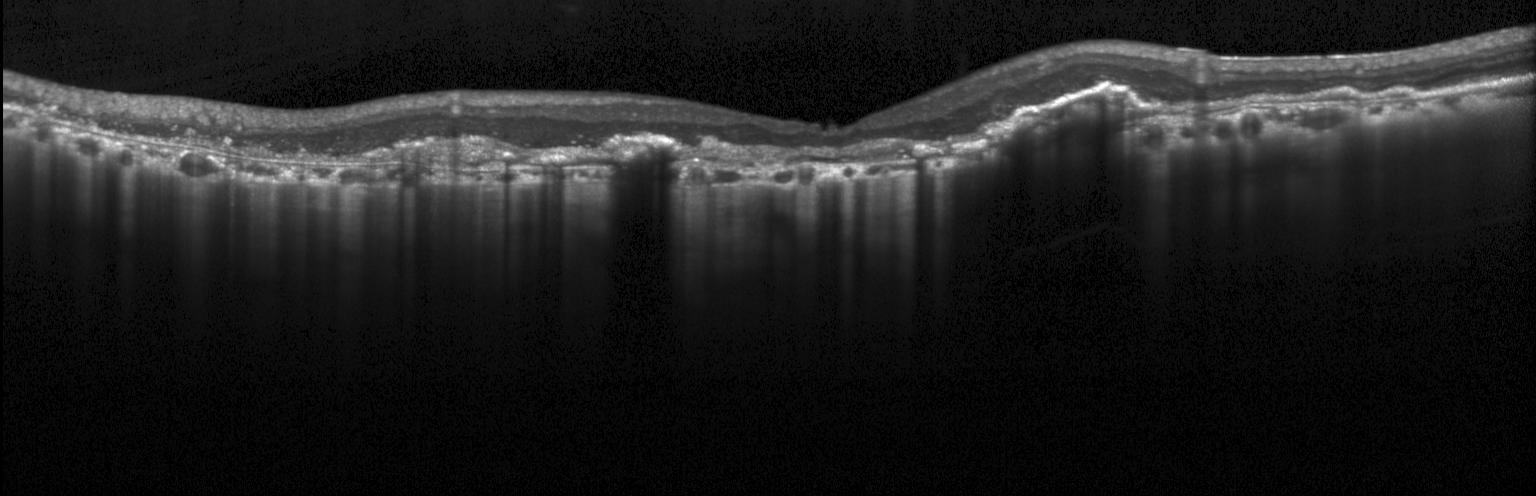
Retinal OCT B-scan. Spectral-domain OCT. This B-scan demonstrates CNV.